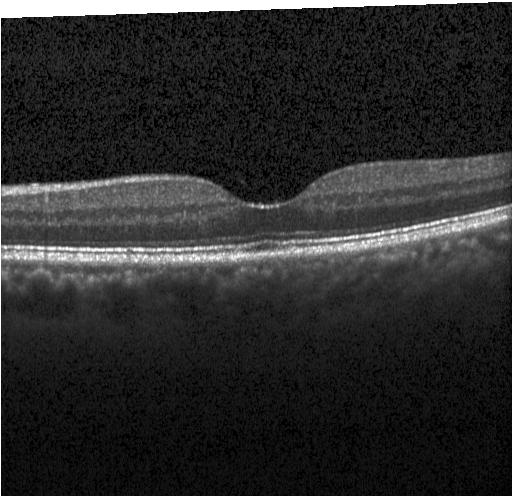
Retinal OCT cross-section showing no evidence of choroidal neovascularization, diabetic macular edema, or drusen.